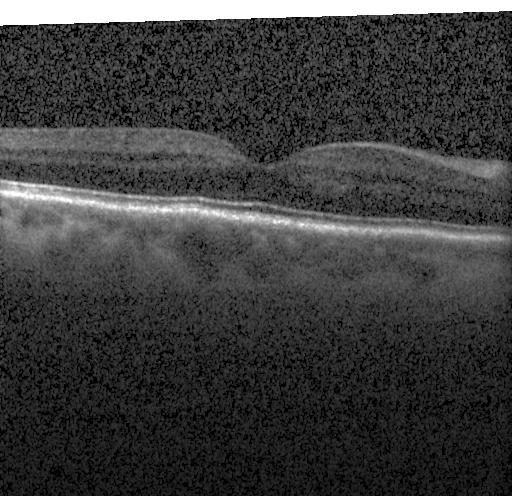
Finding: no evidence of CNV, DME, or drusen.